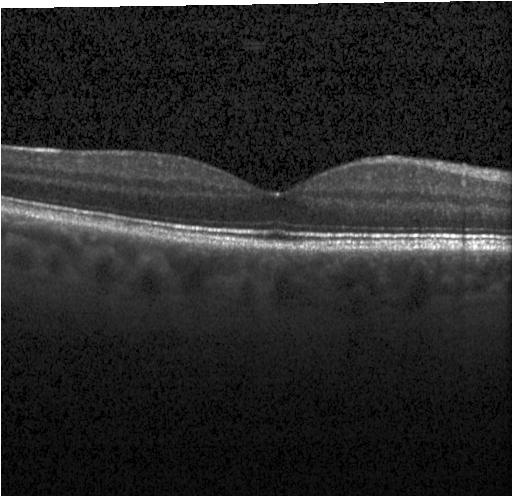
Retinal OCT cross-section, fovea-centered, spectral-domain OCT
Assessment: no choroidal neovascularization, no diabetic macular edema, and no drusen.